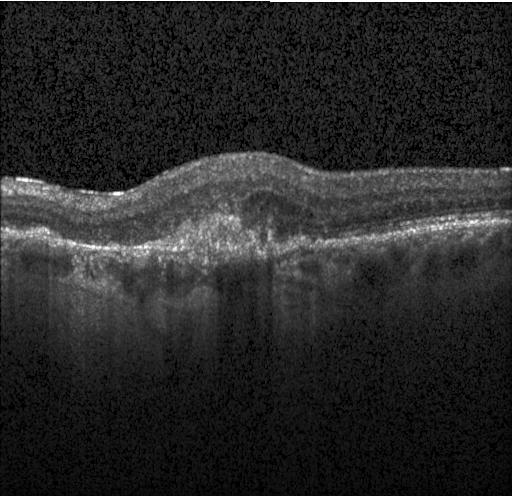
Finding: a choroidal neovascular membrane.